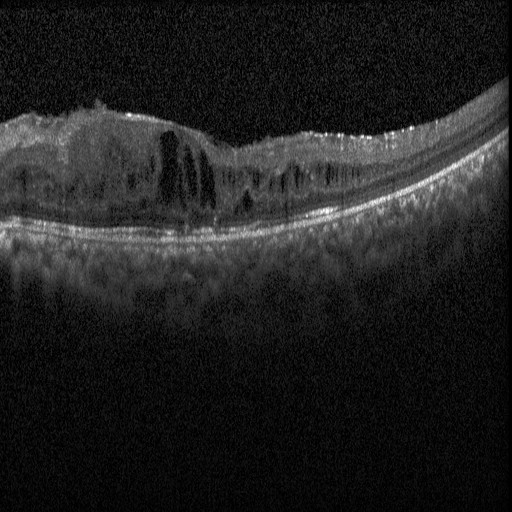

Finding: DME.